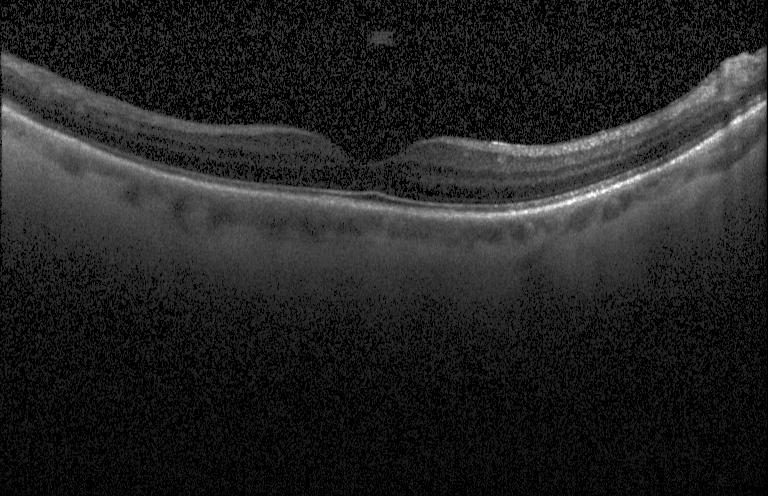 Retinal OCT cross-section.
Impression: no choroidal neovascularization, diabetic macular edema, or drusen.